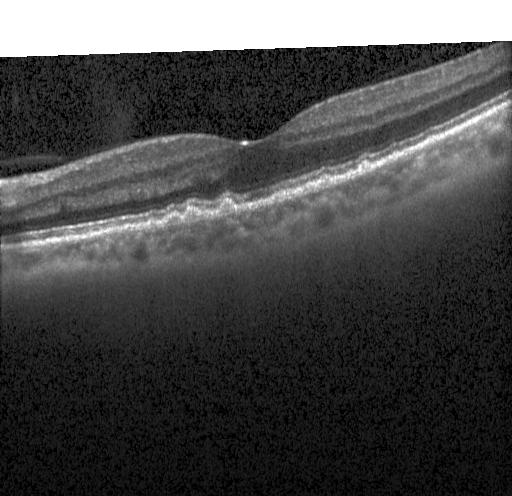
Diagnosis: drusen.